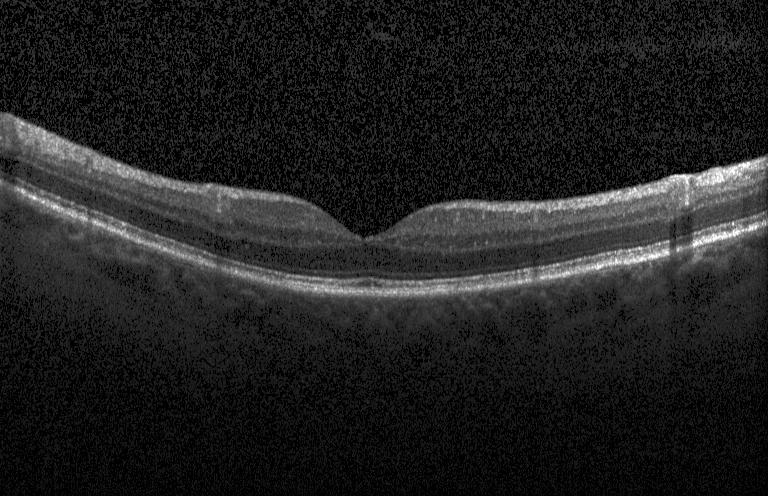

Spectral-domain OCT, retinal OCT cross-section
Diagnosis: no CNV, no DME, and no drusen.